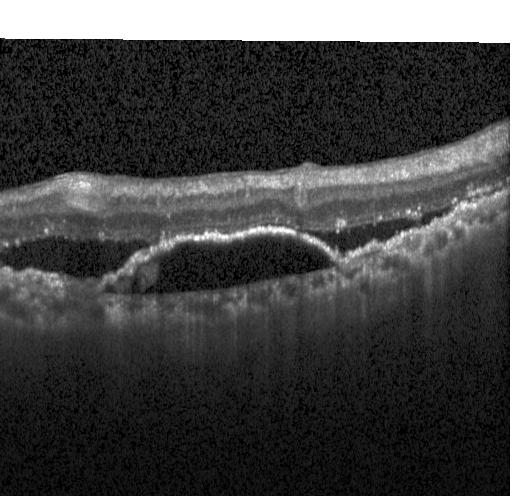 Optical coherence tomography B-scan, horizontal scan through the fovea, SD-OCT — A choroidal neovascular membrane.